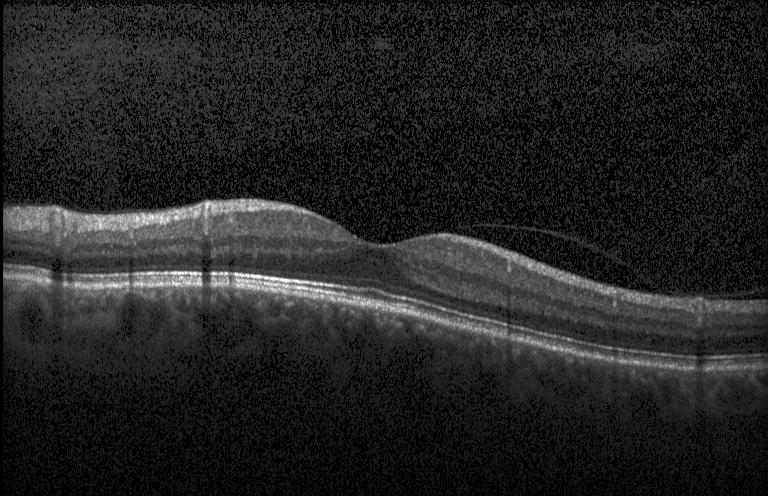

This B-scan demonstrates no evidence of choroidal neovascularization, diabetic macular edema, or drusen.